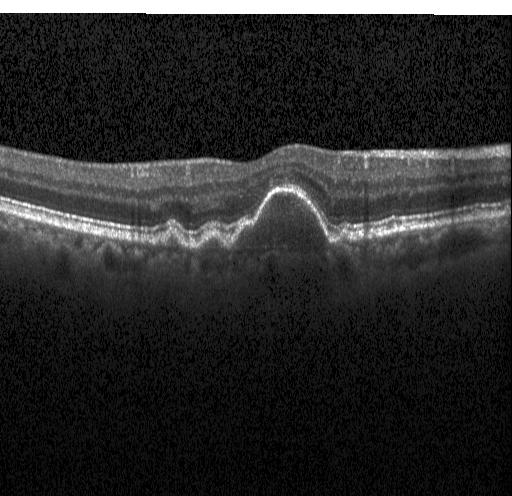 Optical coherence tomography B-scan
Diagnosis: multiple drusen.